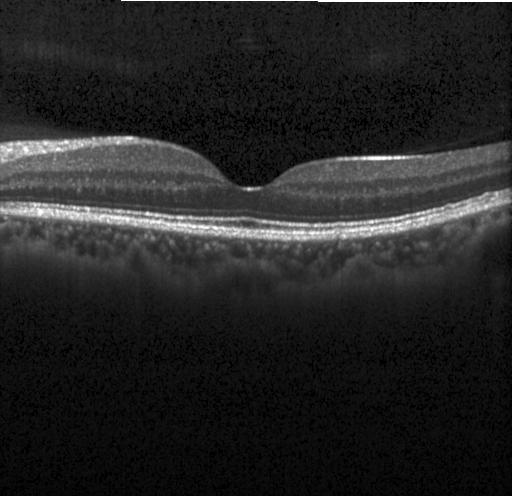 SD-OCT; retinal OCT cross-section; horizontal scan through the fovea; acquired on a Heidelberg Spectralis.
The scan shows no CNV, DME, or drusen.